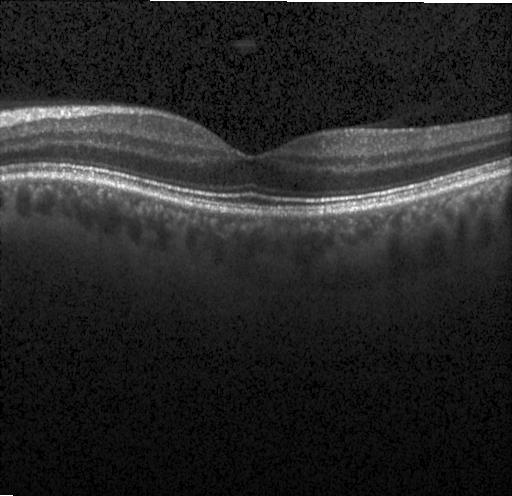

Assessment: neither choroidal neovascularization, diabetic macular edema, nor drusen.